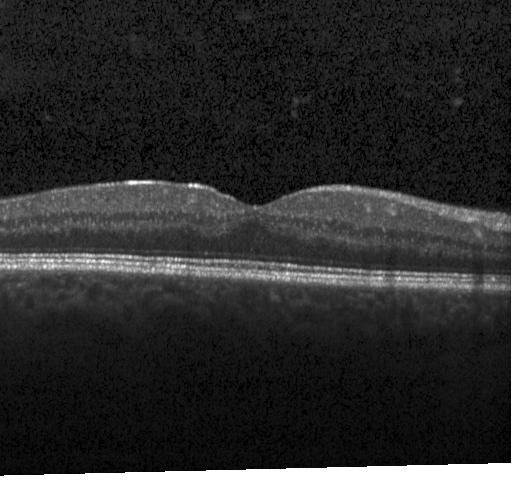

Fovea-centered · SD-OCT · optical coherence tomography B-scan
The scan shows no CNV, no DME, and no drusen.